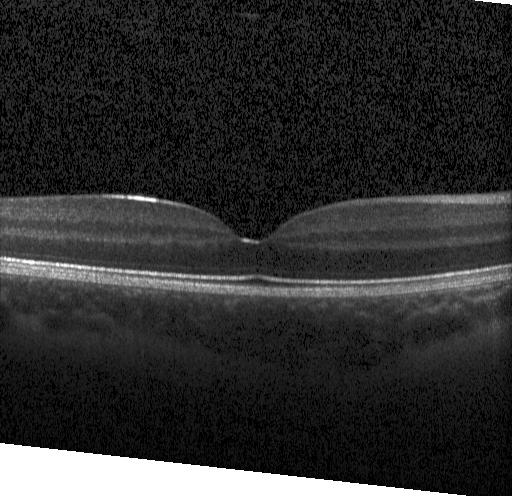

Fovea-centered, retinal OCT B-scan — Impression: no choroidal neovascularization, diabetic macular edema, or drusen.